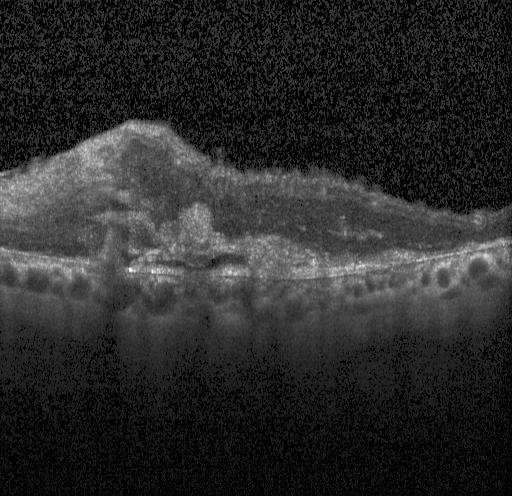
Heidelberg Spectralis. SD-OCT. Retinal OCT B-scan. Centered on the fovea
Impression: a choroidal neovascular membrane.